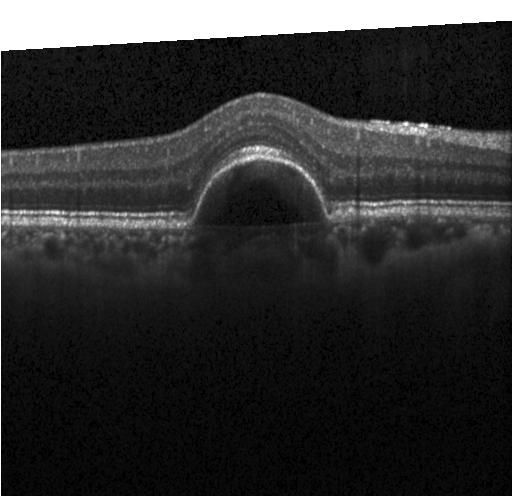 Instrument: Heidelberg Spectralis. OCT B-scan — Impression: CNV.